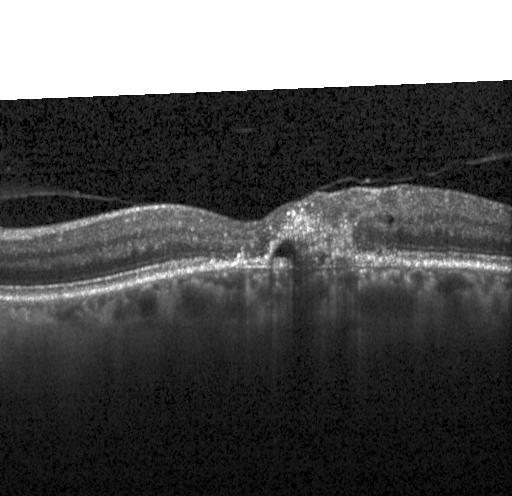
SD-OCT, OCT B-scan. Macular OCT: CNV.